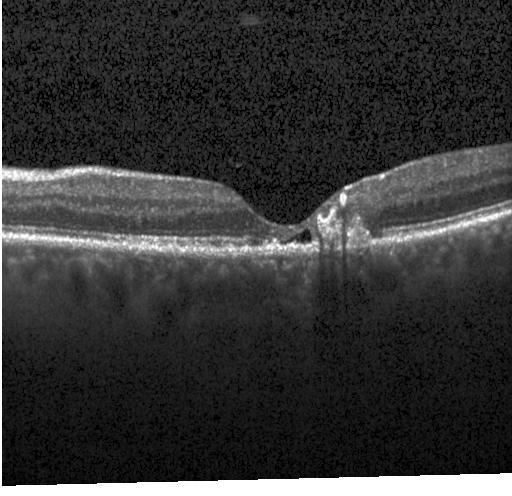

OCT finding: a choroidal neovascular membrane.